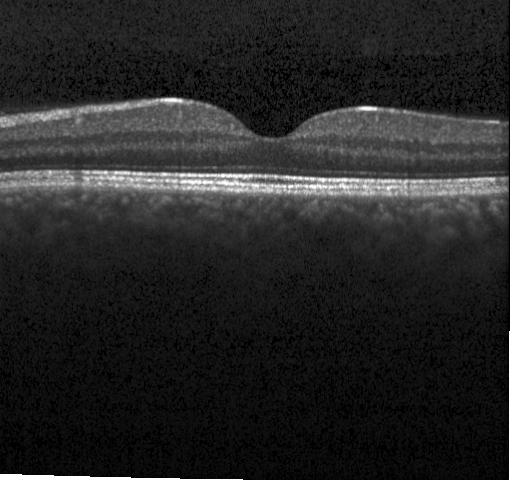

Diagnosis: no choroidal neovascularization, no diabetic macular edema, and no drusen.